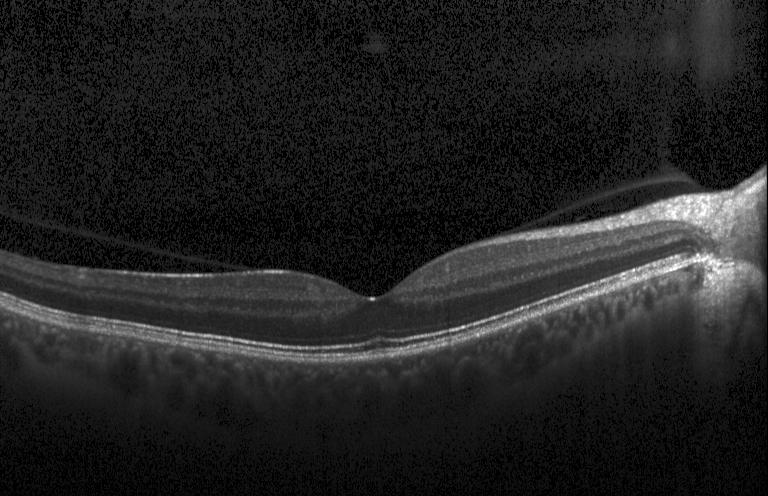
Retinal OCT cross-section, acquired on a Heidelberg Spectralis.
Dx: no choroidal neovascularization, diabetic macular edema, or drusen.